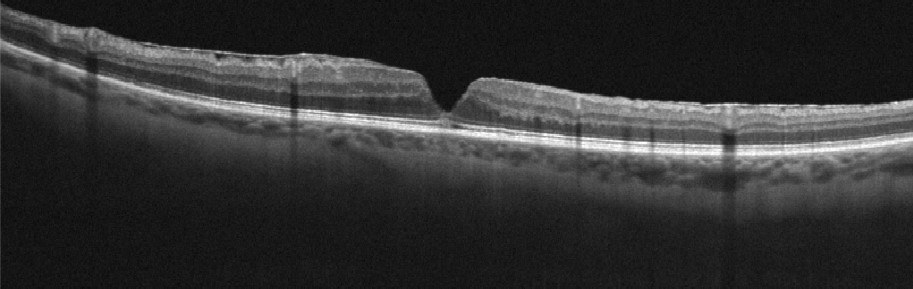

Acquired on an Optovue Avanti RTVue XR. OCT B-scan. Diagnosis: epiretinal membrane.